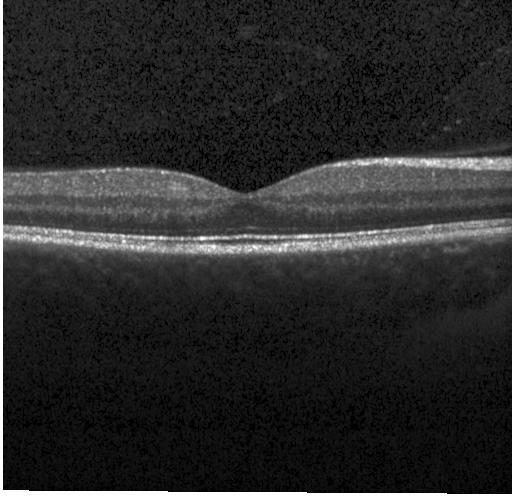

OCT line scan, spectral-domain OCT. The scan shows no evidence of choroidal neovascularization, diabetic macular edema, or drusen.